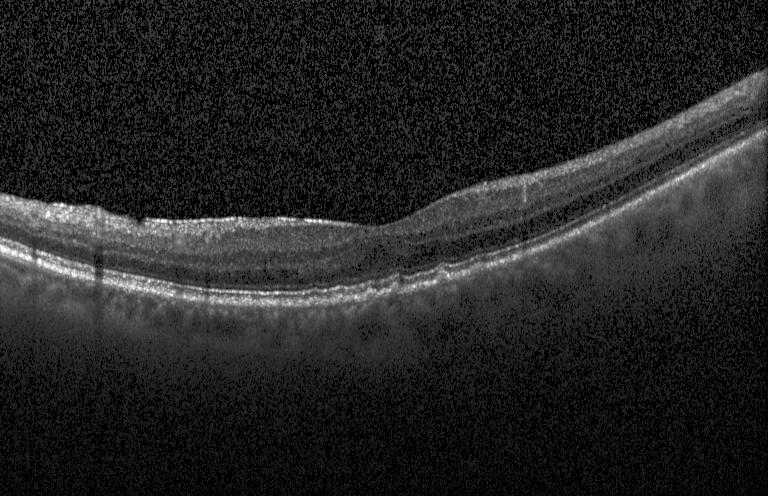
Optical coherence tomography B-scan — Assessment: drusen.